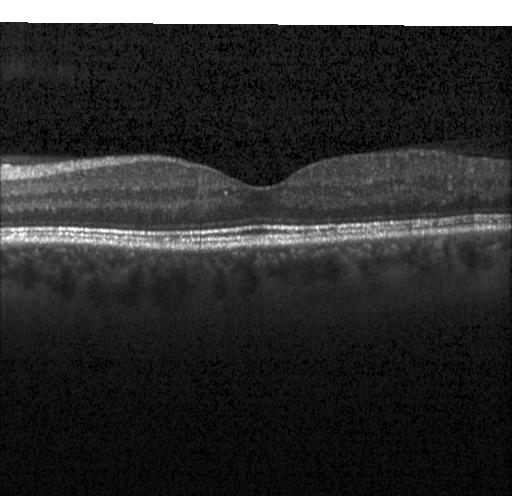

Retinal OCT cross-section.
Dx: neither CNV, DME, nor drusen.